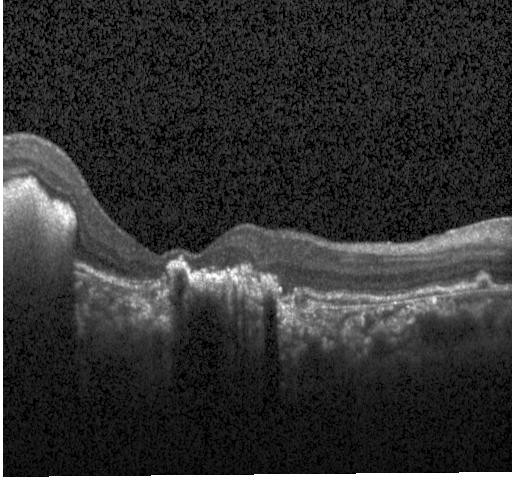 Fovea-centered · Heidelberg Spectralis · retinal OCT cross-section.
Assessment: a choroidal neovascular membrane.